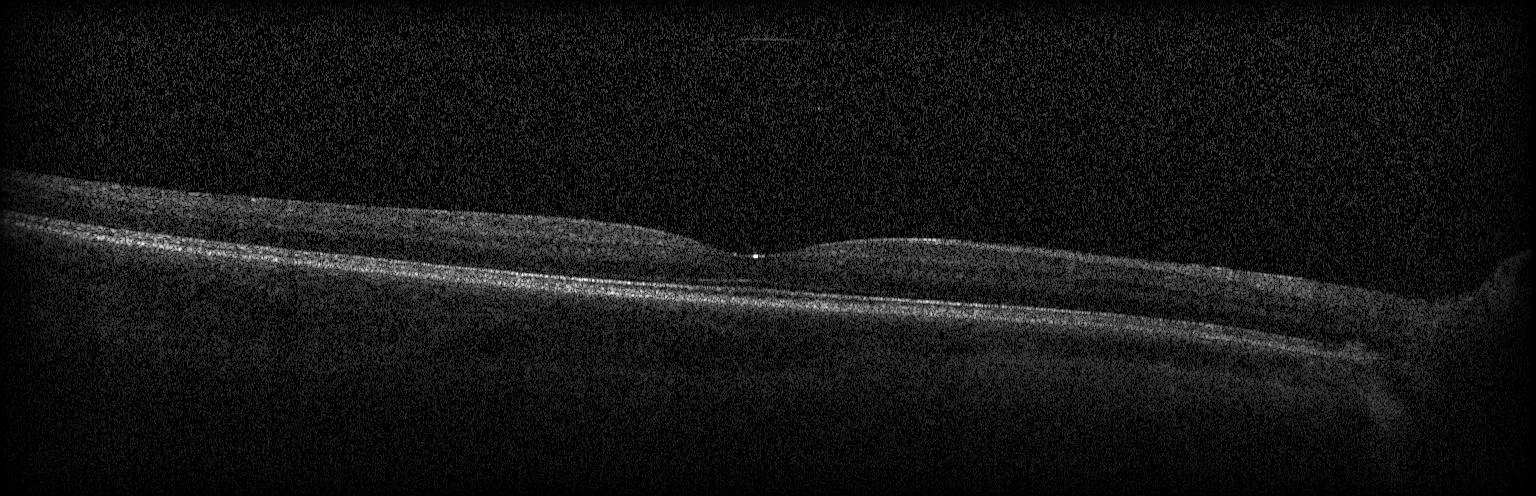 Heidelberg Spectralis OCT system. Through the macula. Spectral-domain OCT. OCT line scan — Diagnosis: no CNV, DME, or drusen.